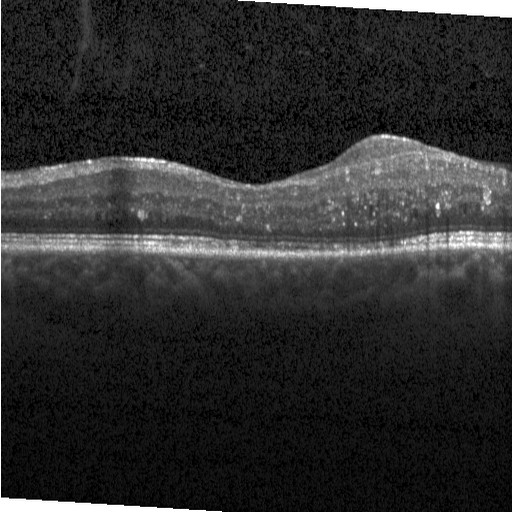
Impression: diabetic macular edema (DME).